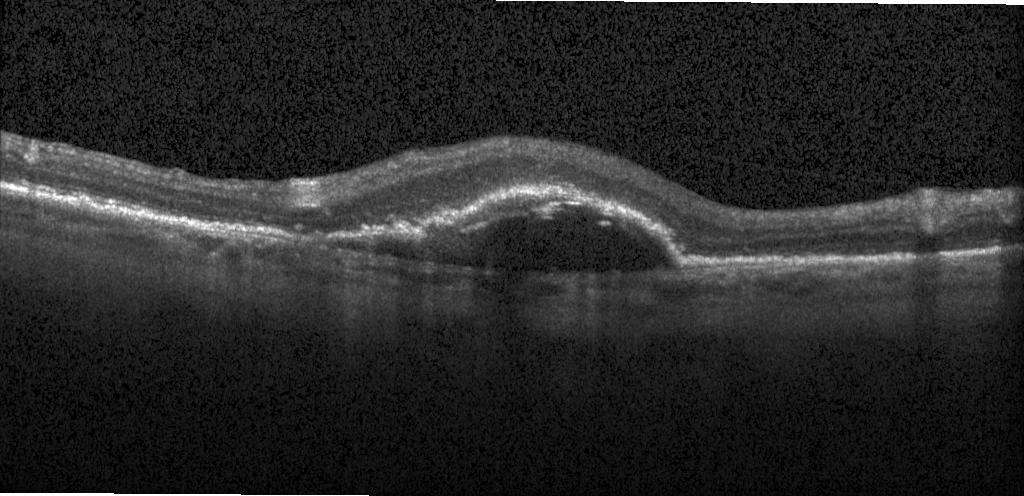

OCT B-scan.
Finding: choroidal neovascularization.